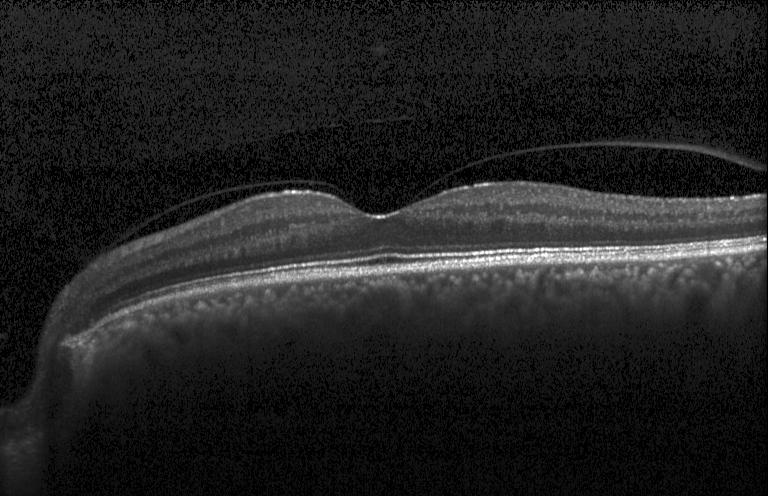

OCT B-scan showing no choroidal neovascularization, diabetic macular edema, or drusen.